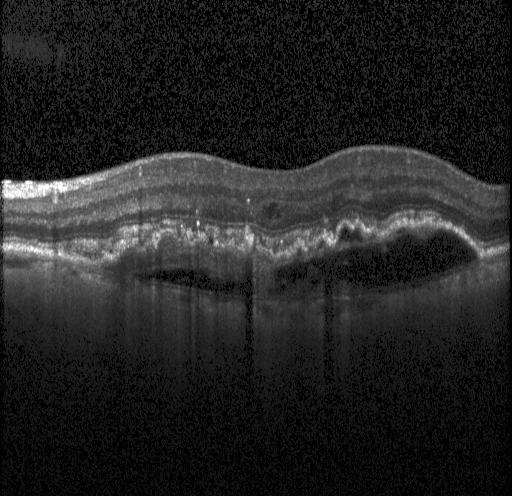 Finding: CNV.